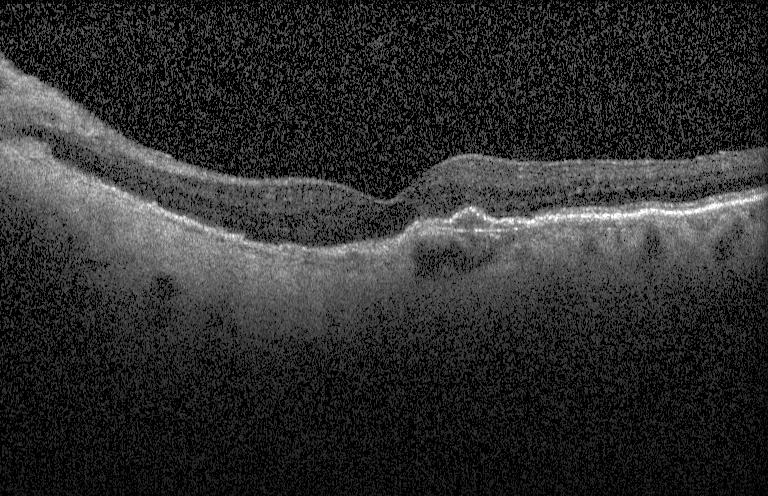
Retinal OCT B-scan. Impression: a choroidal neovascular membrane.